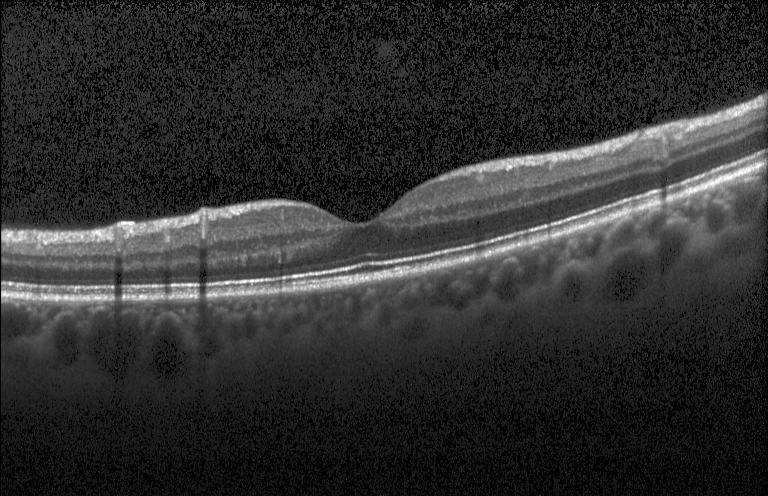
OCT line scan; macular scan
OCT finding: neither choroidal neovascularization, diabetic macular edema, nor drusen.